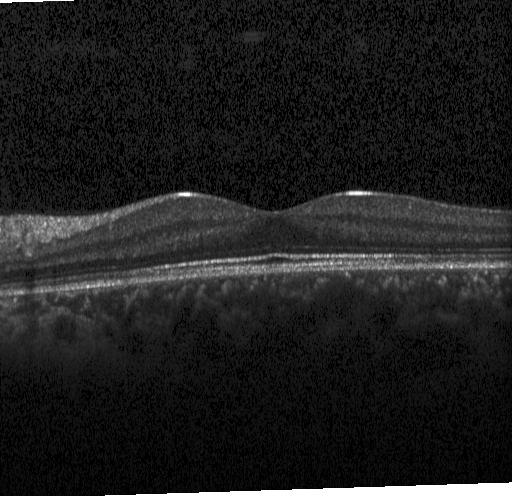
Optical coherence tomography B-scan. Through the macula. Acquired on a Heidelberg Spectralis. The scan shows no evidence of choroidal neovascularization, diabetic macular edema, or drusen.